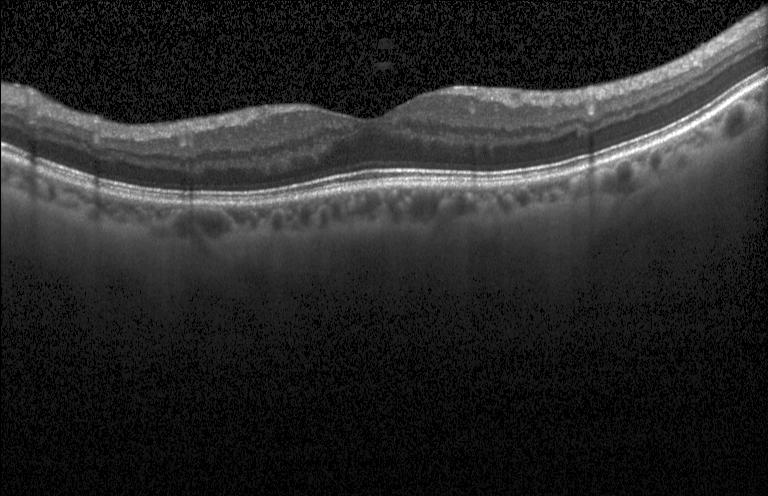

Heidelberg Spectralis. Macular scan. OCT B-scan.
Impression: no choroidal neovascularization, no diabetic macular edema, and no drusen.